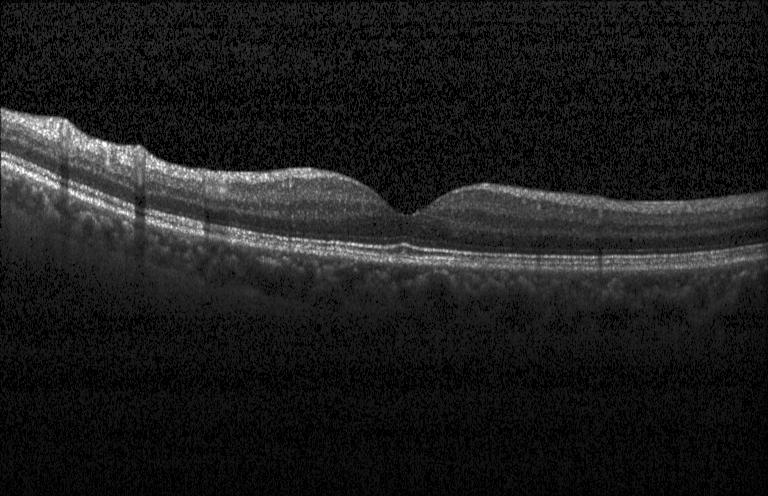
Finding: neither CNV, DME, nor drusen.